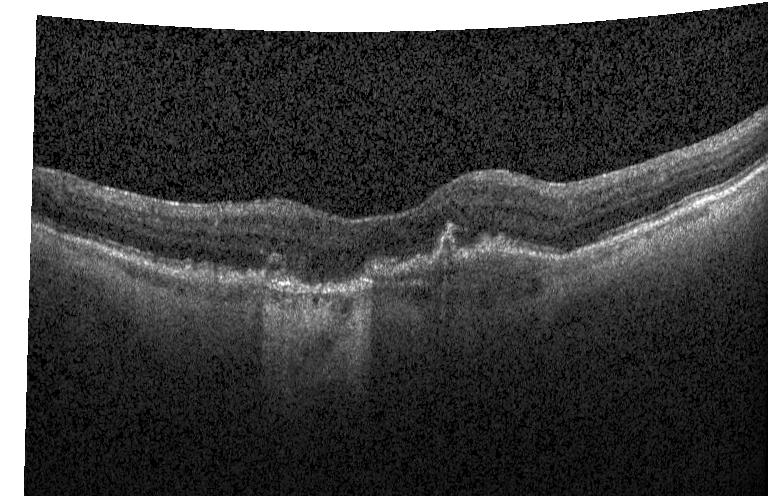
Macular scan, retinal OCT cross-section, SD-OCT, Heidelberg Spectralis OCT system — Macular OCT: a choroidal neovascular membrane.